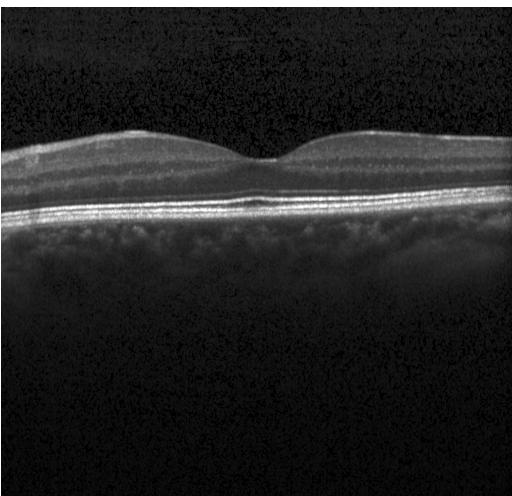
Optical coherence tomography B-scan · acquired on a Heidelberg Spectralis · fovea-centered · SD-OCT — Impression: no evidence of CNV, DME, or drusen.